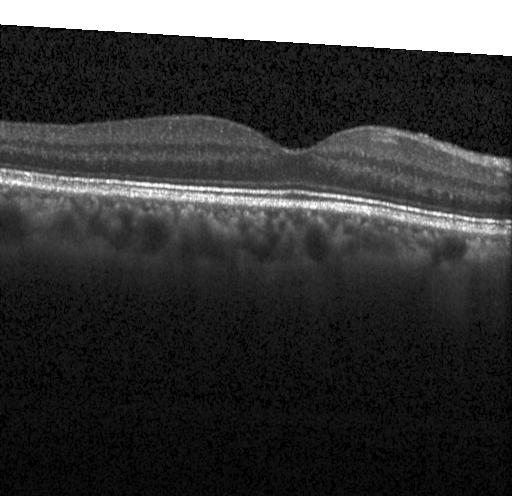

Finding: neither choroidal neovascularization, diabetic macular edema, nor drusen.